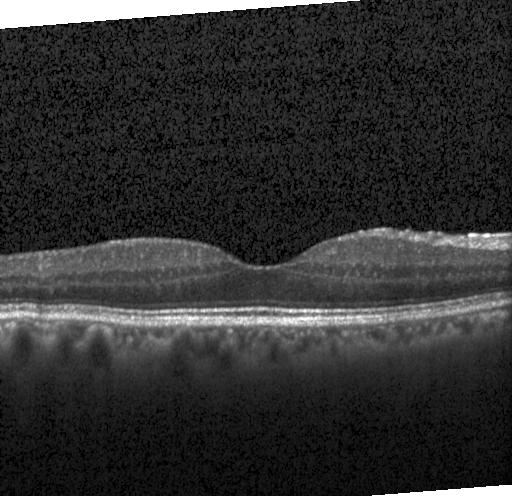

Assessment: no CNV, DME, or drusen.